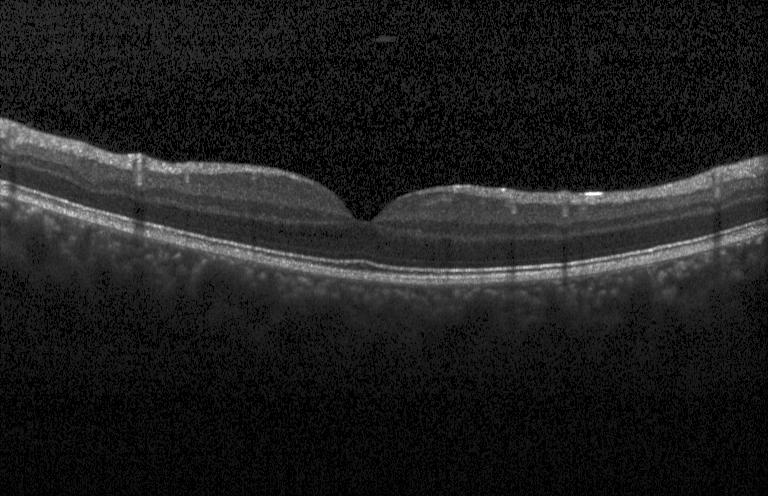

Finding: no evidence of choroidal neovascularization, diabetic macular edema, or drusen.